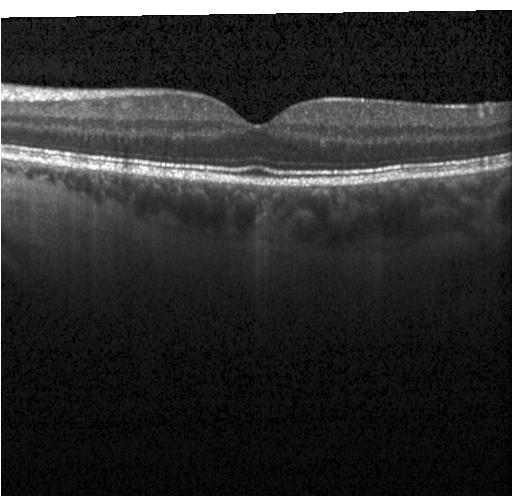 Dx: no CNV, no DME, and no drusen.